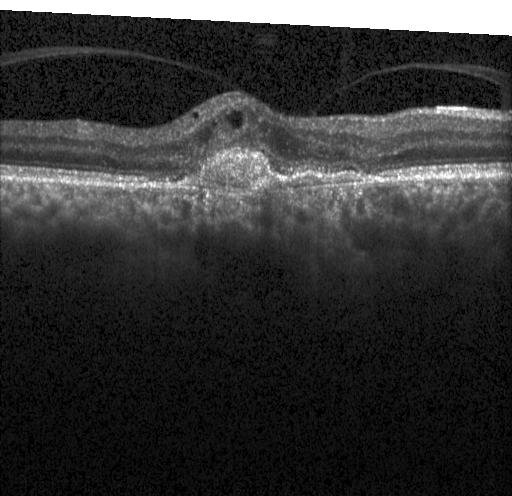 Finding: CNV.